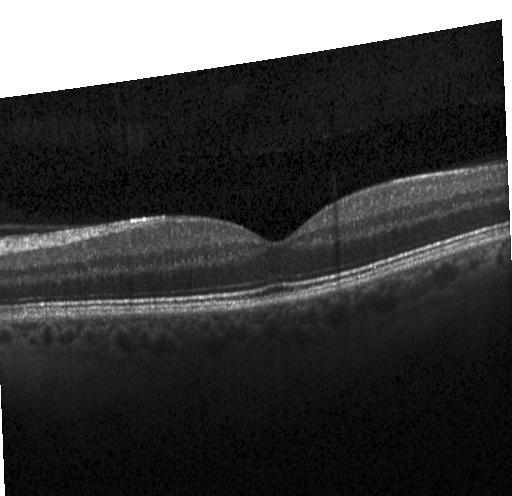

Heidelberg Spectralis. OCT B-scan.
This B-scan demonstrates no CNV, DME, or drusen.